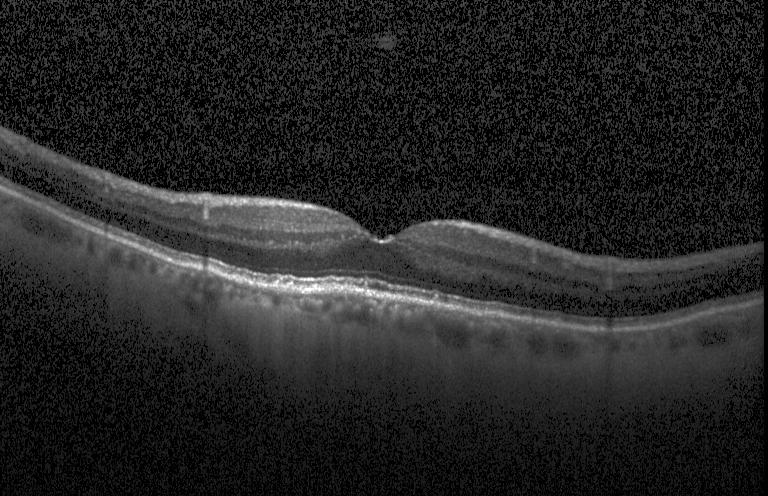

Assessment: multiple drusen.